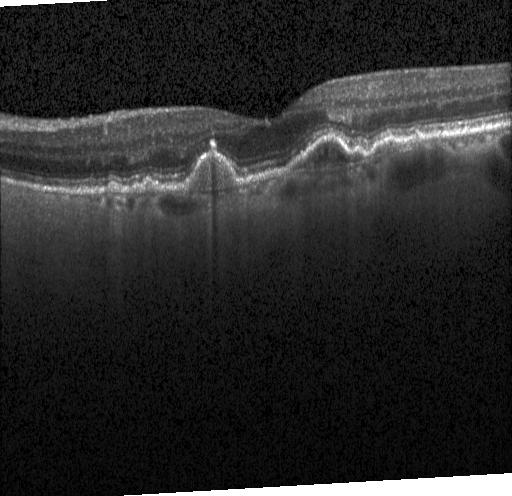 Heidelberg Spectralis, retinal OCT B-scan, centered on the fovea. Finding: choroidal neovascularization.